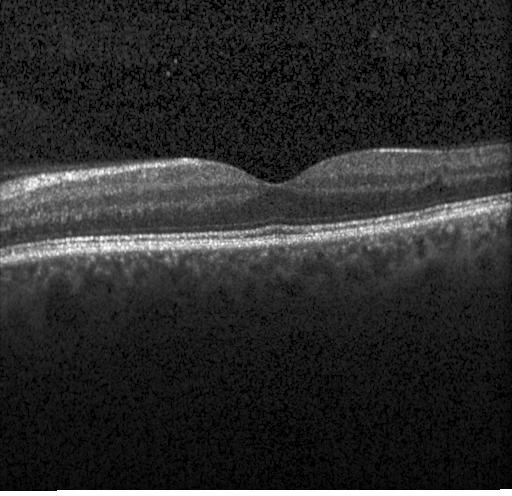

Diagnosis: no evidence of choroidal neovascularization, diabetic macular edema, or drusen.